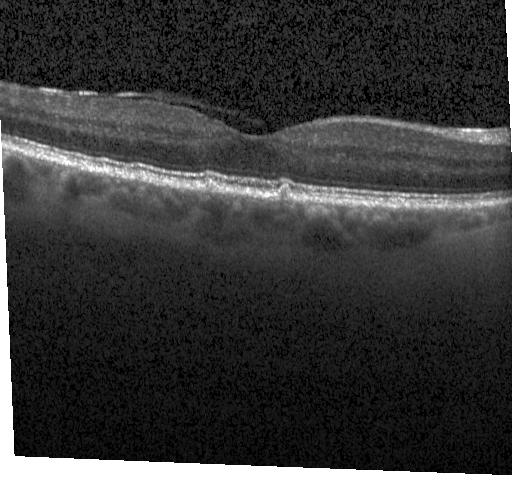 Spectral-domain OCT · acquired on a Heidelberg Spectralis · optical coherence tomography B-scan · macular scan — Diagnosis: drusen.